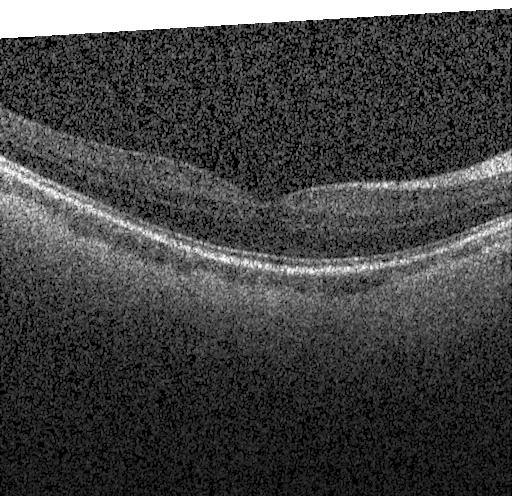

OCT B-scan showing no evidence of choroidal neovascularization, diabetic macular edema, or drusen.